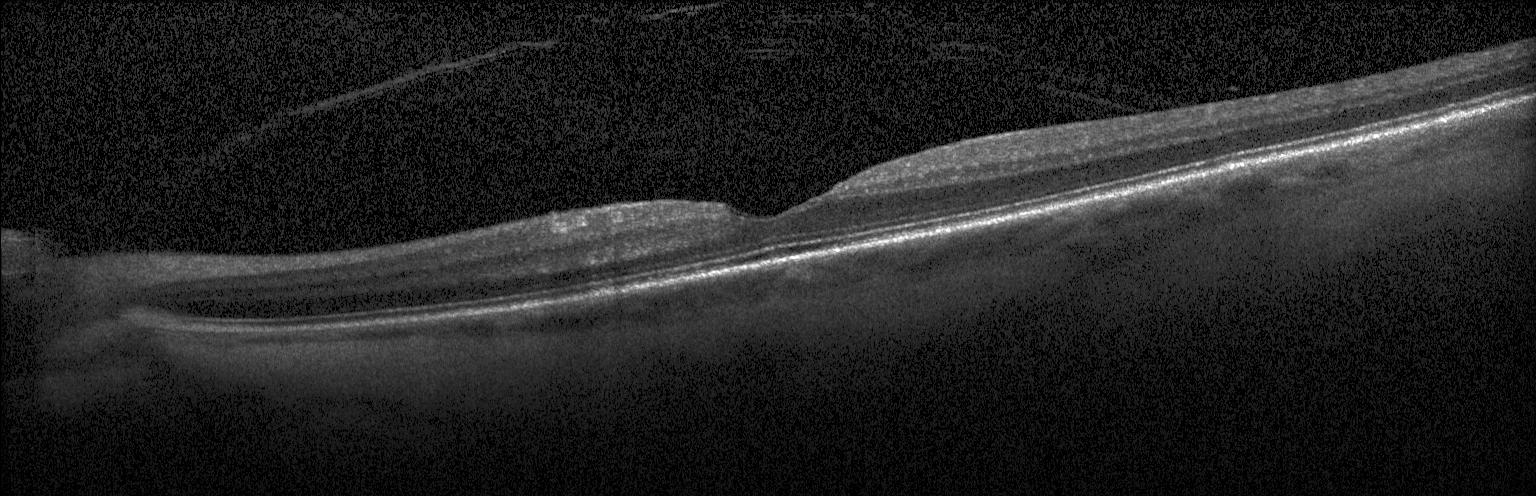
OCT scan showing no choroidal neovascularization, no diabetic macular edema, and no drusen.